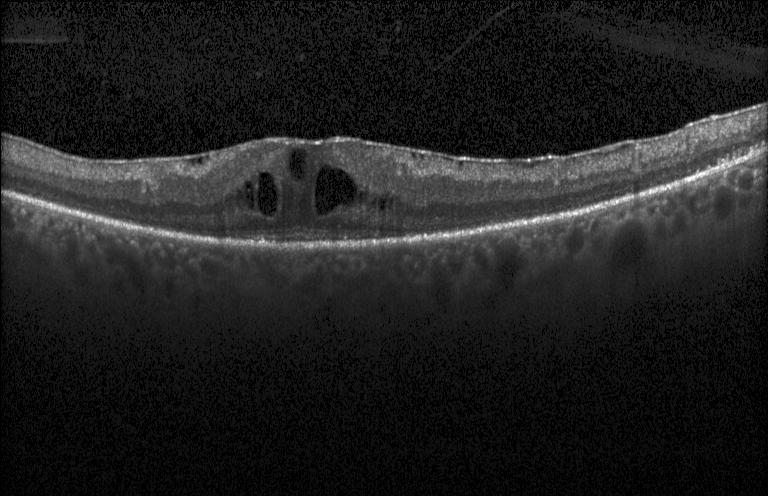 Spectral-domain OCT B-scan: diabetic macular edema.